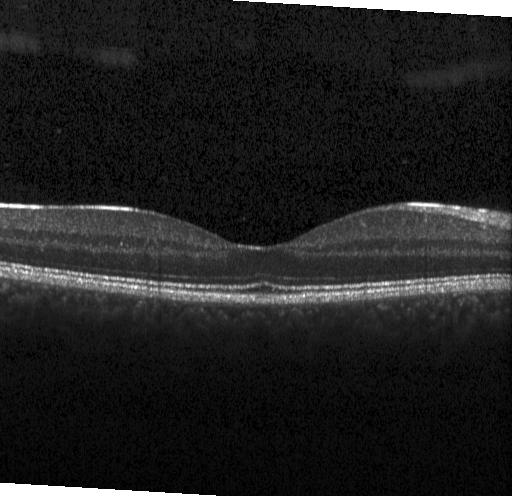

Spectral-domain optical coherence tomography. Acquired on a Heidelberg Spectralis. Retinal OCT cross-section. Dx: no choroidal neovascularization, diabetic macular edema, or drusen.